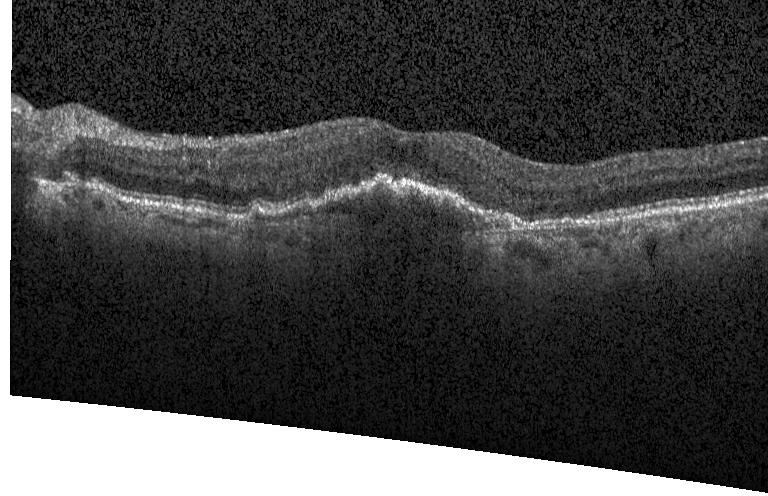 Impression: a choroidal neovascular membrane.